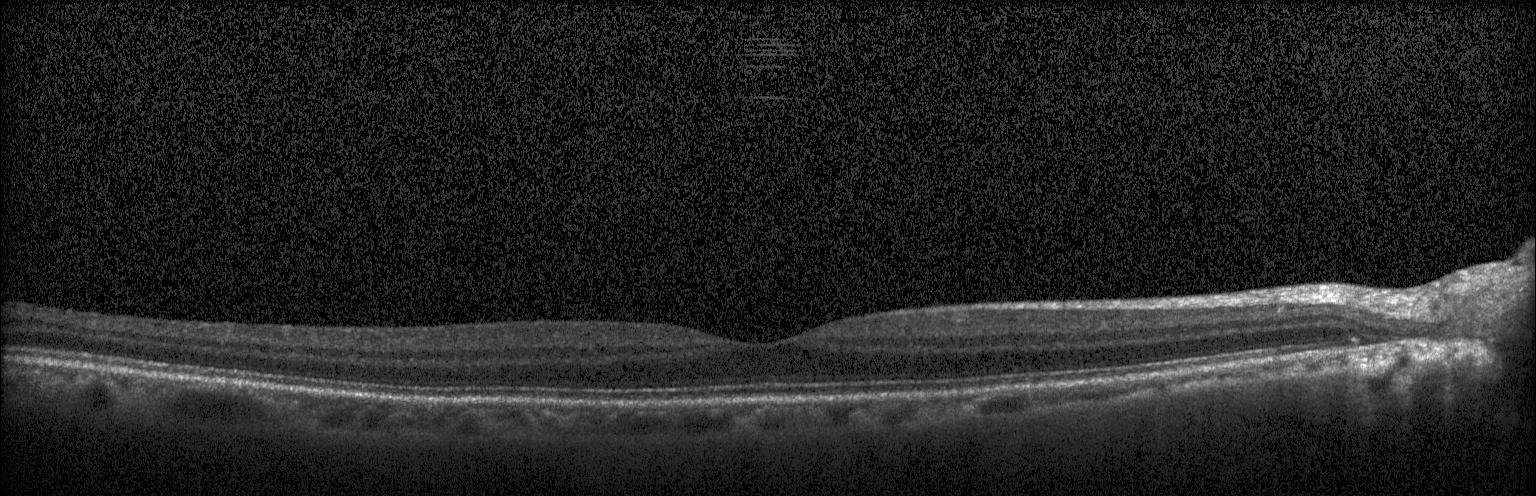
OCT line scan; centered on the fovea — This B-scan demonstrates no choroidal neovascularization, no diabetic macular edema, and no drusen.